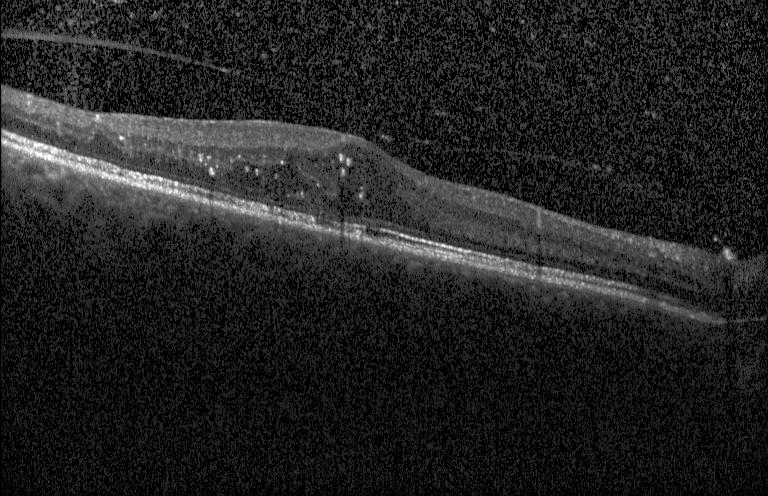

The scan shows diabetic macular edema (DME).